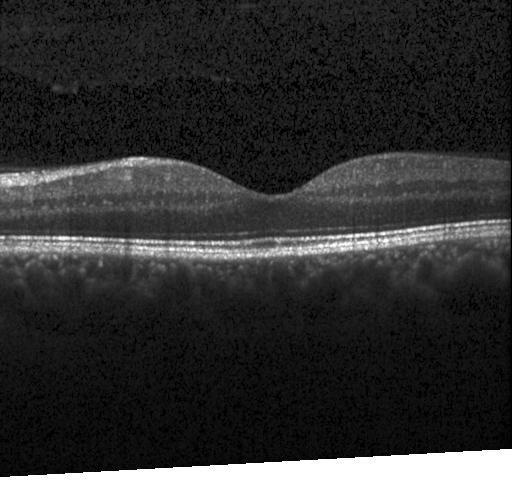 OCT scan showing no choroidal neovascularization, no diabetic macular edema, and no drusen.